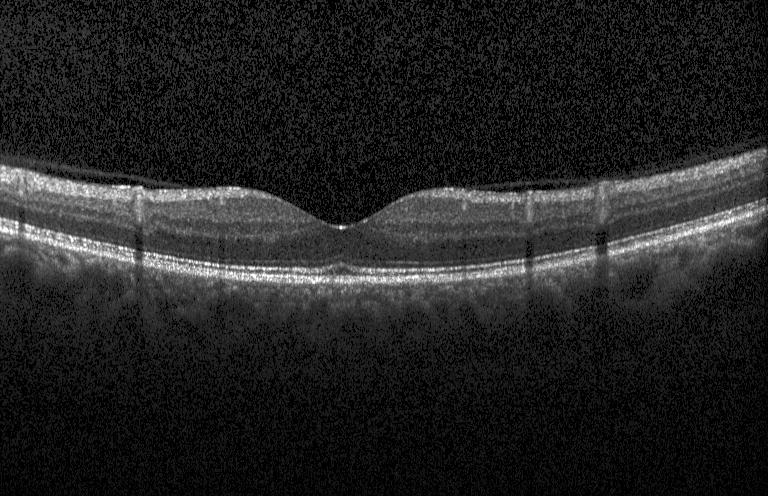

Optical coherence tomography scan
Impression: no choroidal neovascularization, diabetic macular edema, or drusen.